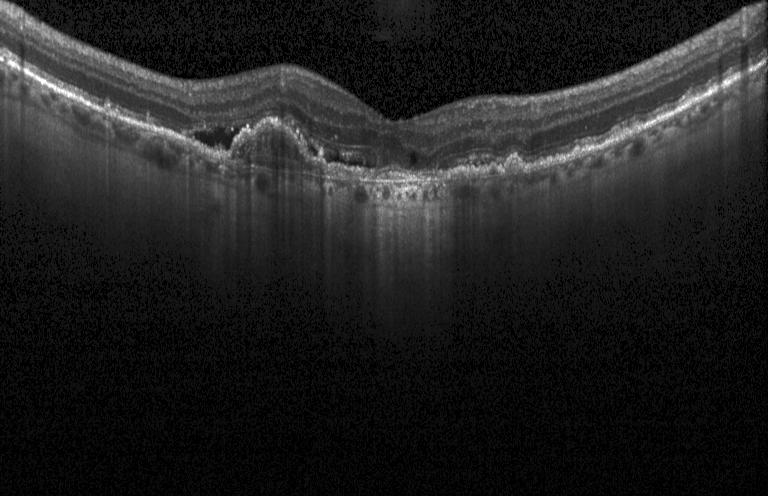 Assessment: choroidal neovascularization.